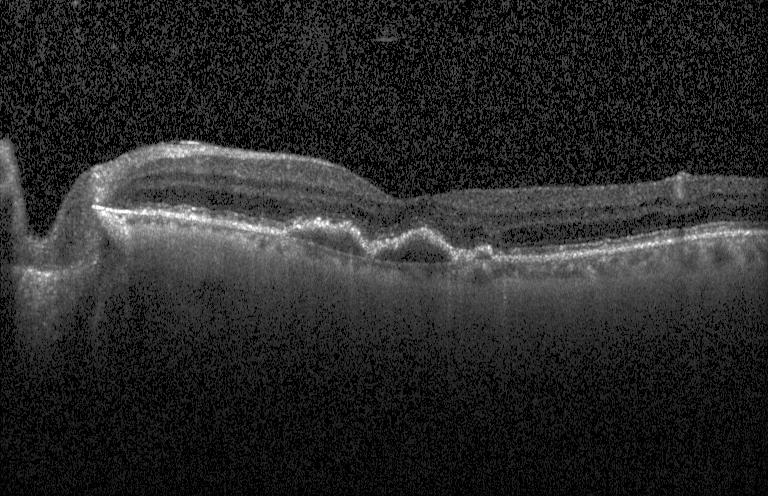

Spectral-domain OCT B-scan: a choroidal neovascular membrane.